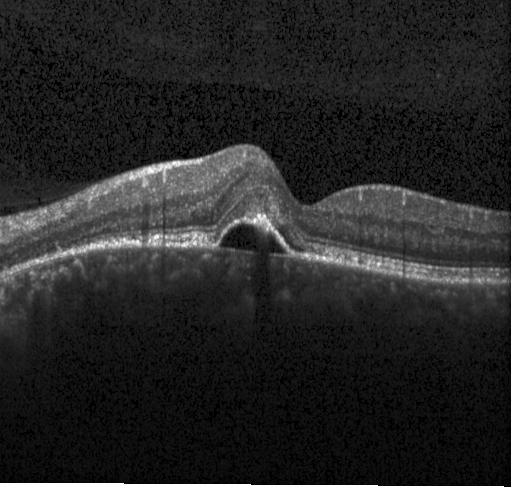

Centered on the fovea, retinal OCT B-scan.
Assessment: a choroidal neovascular membrane.